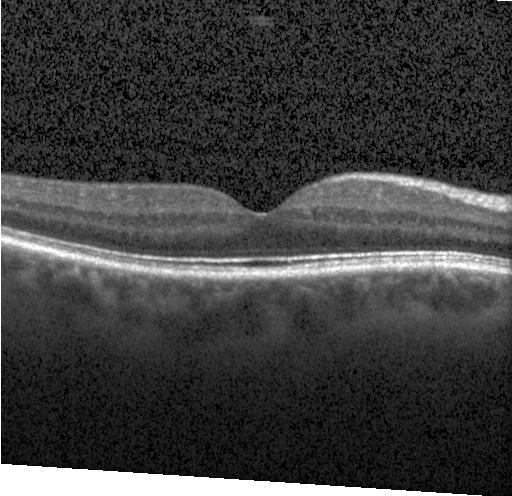

Spectral-domain optical coherence tomography. OCT B-scan — This B-scan demonstrates no choroidal neovascularization, no diabetic macular edema, and no drusen.